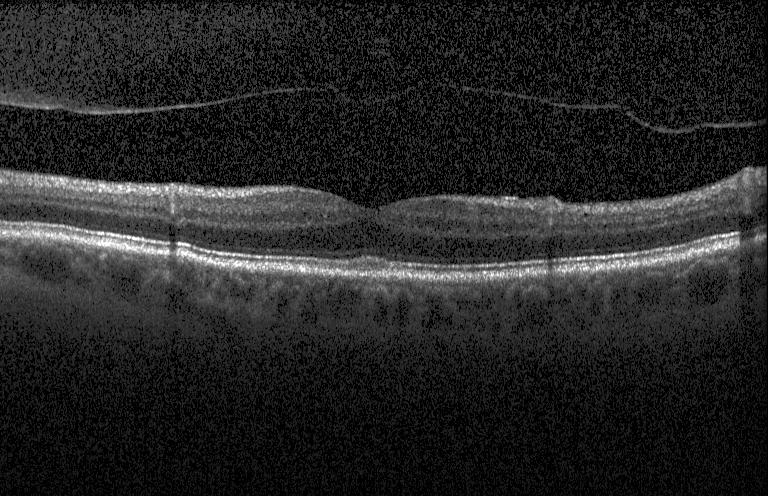

Assessment: no evidence of choroidal neovascularization, diabetic macular edema, or drusen.